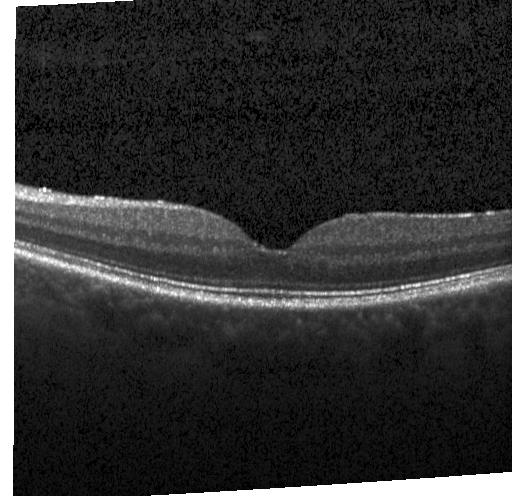 Horizontal scan through the fovea; instrument: Heidelberg Spectralis; spectral-domain optical coherence tomography; OCT B-scan.
Diagnosis: no choroidal neovascularization, no diabetic macular edema, and no drusen.